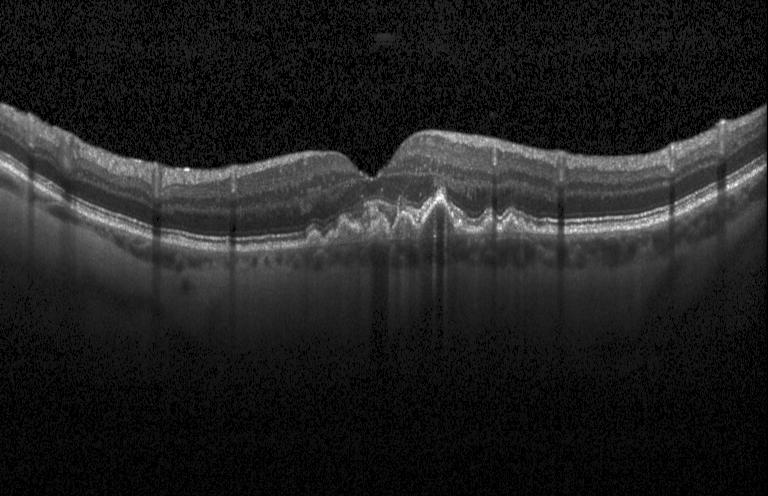 This B-scan demonstrates sub-RPE drusenoid deposits.